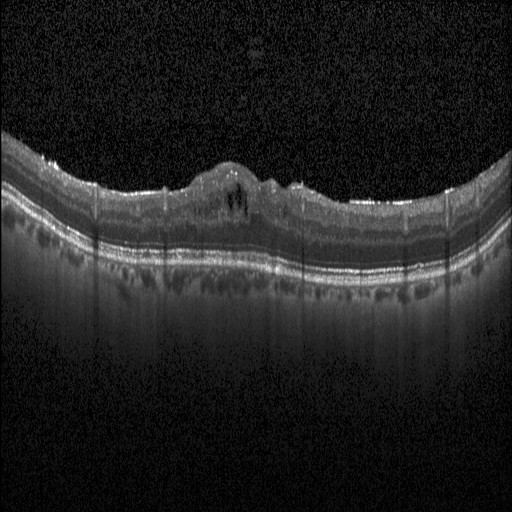

SD-OCT · OCT B-scan · Heidelberg Spectralis OCT system · horizontal scan through the fovea. Finding: diabetic macular edema.